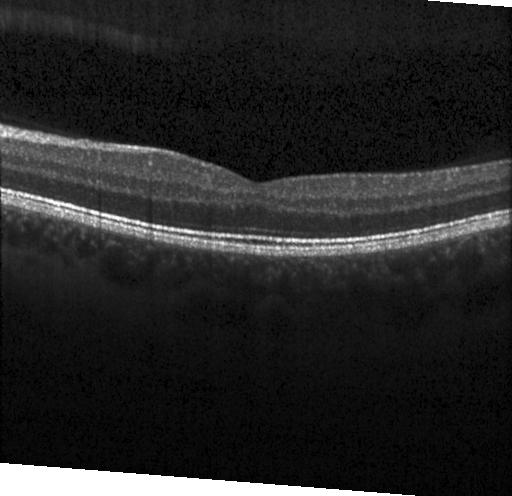 OCT line scan; acquired on a Heidelberg Spectralis; spectral-domain optical coherence tomography
OCT finding: no CNV, DME, or drusen.